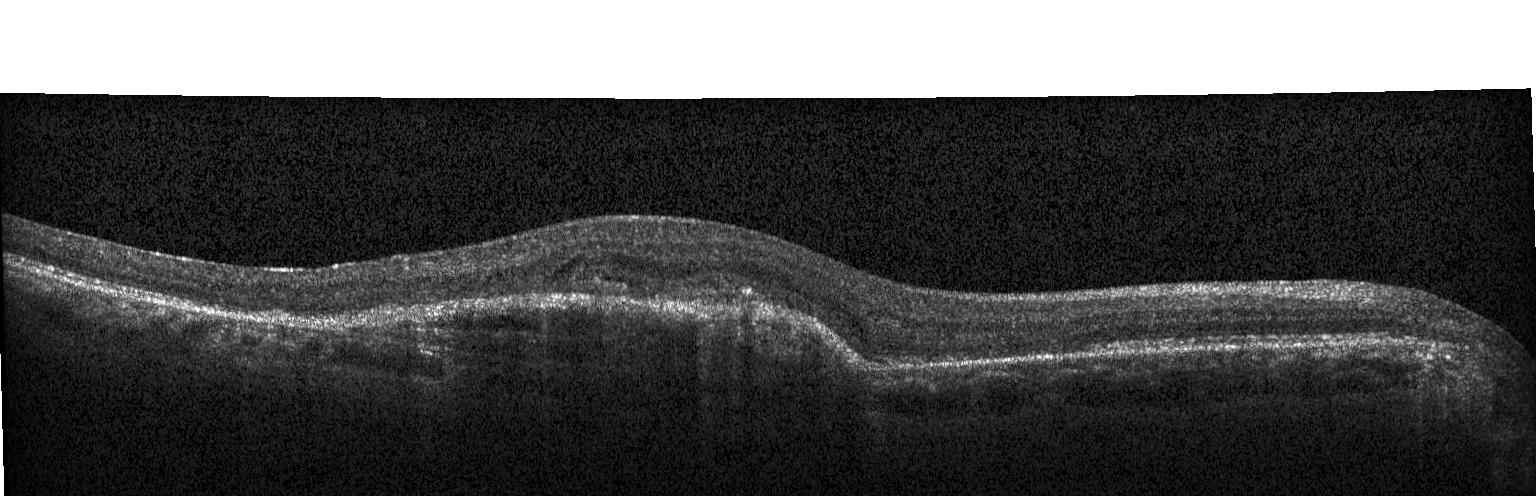
Retinal OCT cross-section showing a choroidal neovascular membrane.